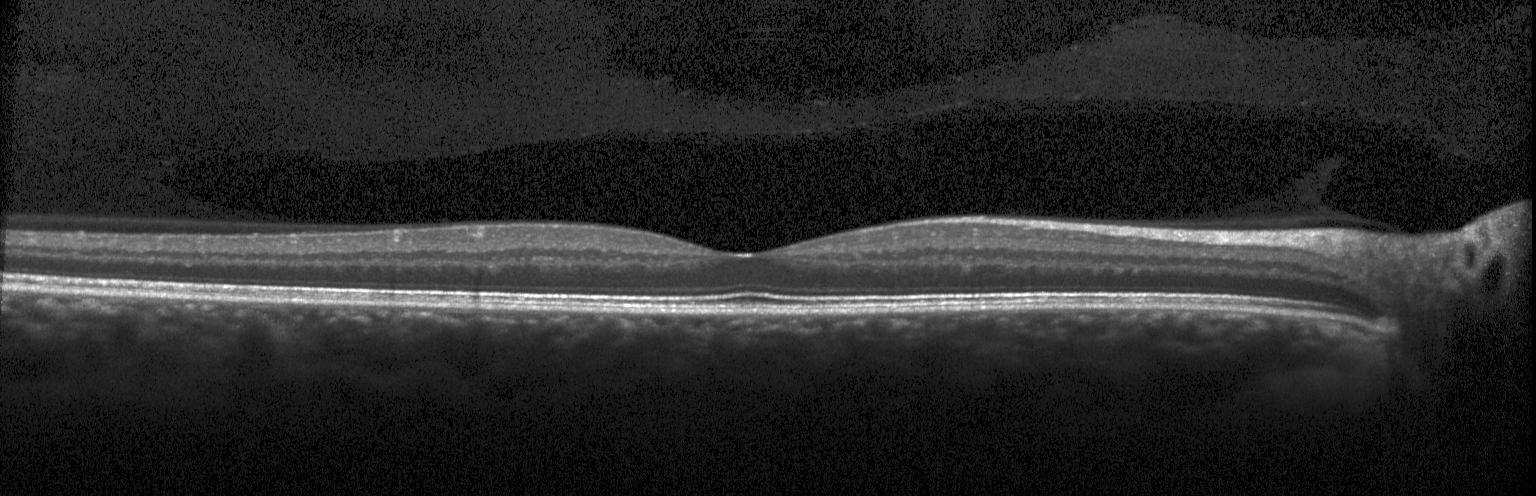 Assessment: neither choroidal neovascularization, diabetic macular edema, nor drusen.